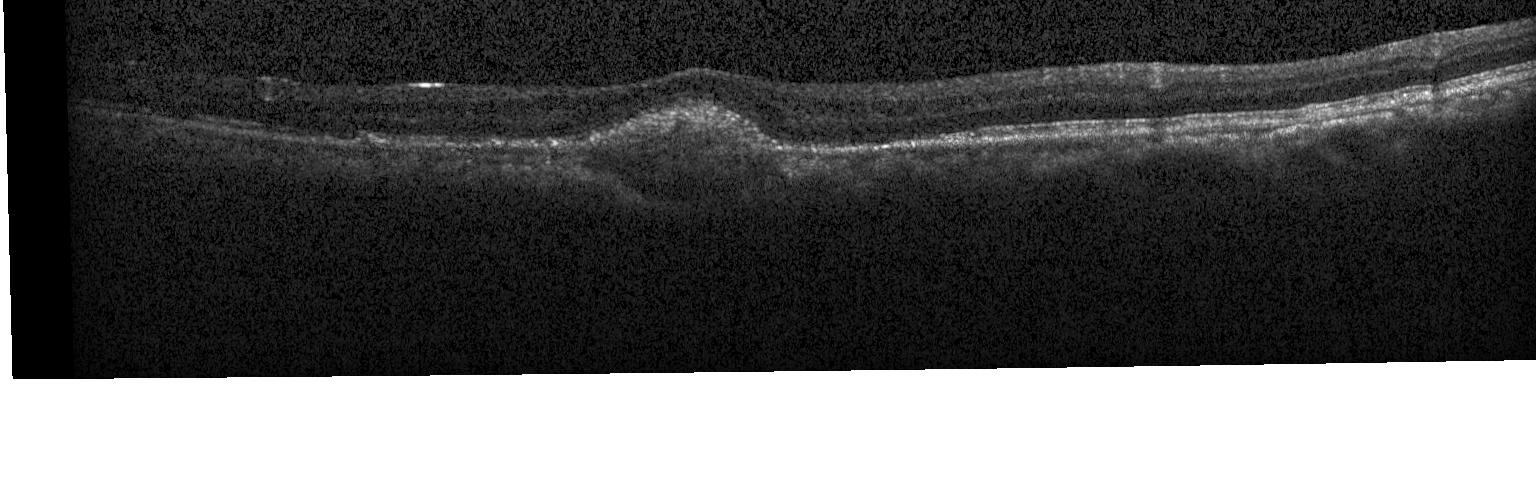
Finding: a choroidal neovascular membrane.